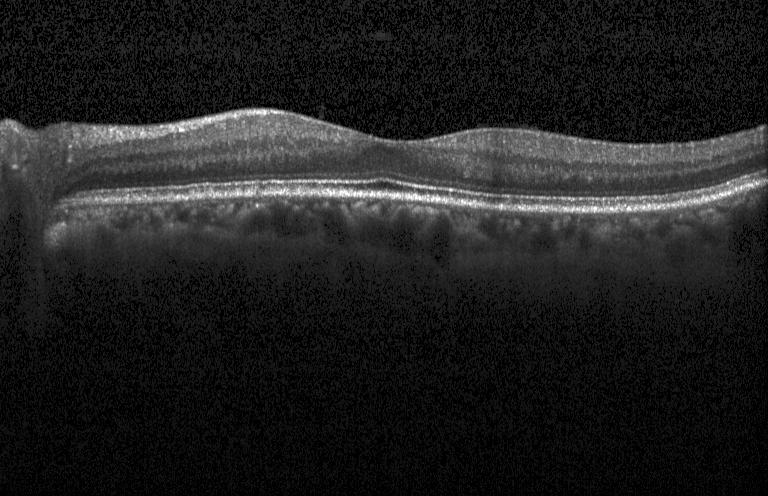 SD-OCT · Heidelberg Spectralis · optical coherence tomography scan
Dx: no evidence of CNV, DME, or drusen.